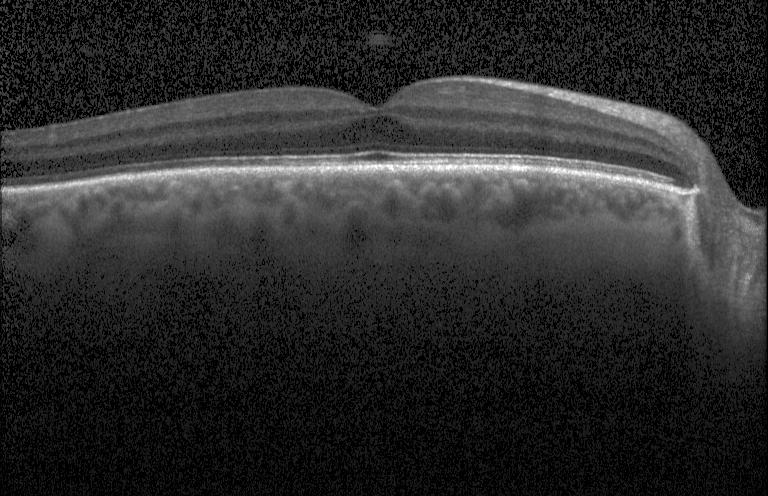 Horizontal scan through the fovea; optical coherence tomography scan; spectral-domain OCT — Macular OCT: neither CNV, DME, nor drusen.